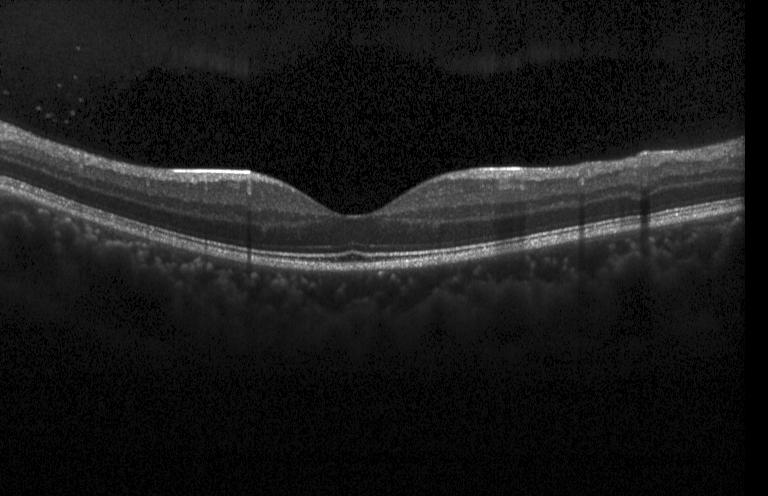
Heidelberg Spectralis · optical coherence tomography B-scan · horizontal scan through the fovea. The scan shows no evidence of choroidal neovascularization, diabetic macular edema, or drusen.